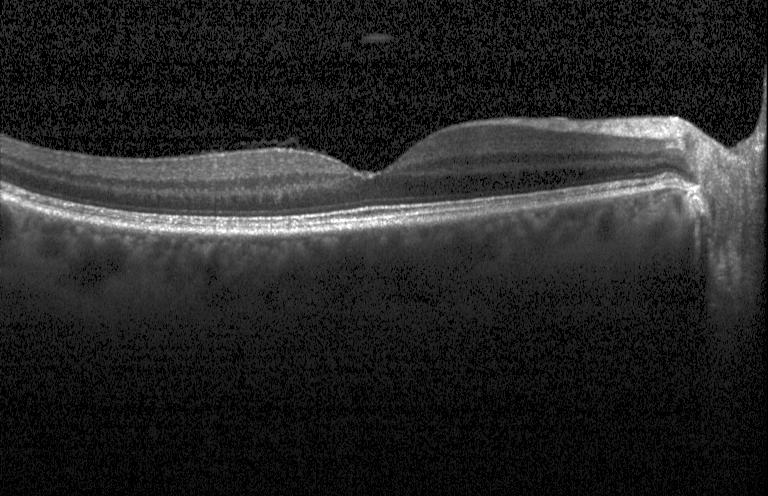
Heidelberg Spectralis. Macular scan. OCT B-scan — This B-scan demonstrates no choroidal neovascularization, no diabetic macular edema, and no drusen.